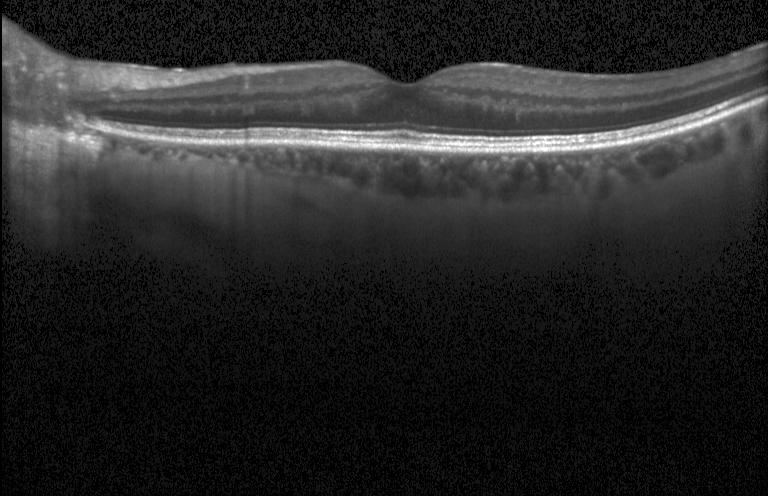 Finding: no choroidal neovascularization, no diabetic macular edema, and no drusen.